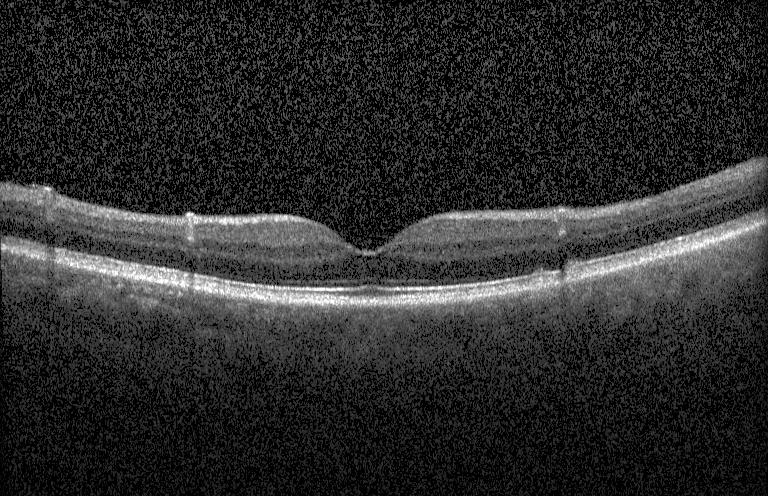
Through the macula. OCT B-scan. Heidelberg Spectralis OCT system
Macular OCT: no choroidal neovascularization, no diabetic macular edema, and no drusen.